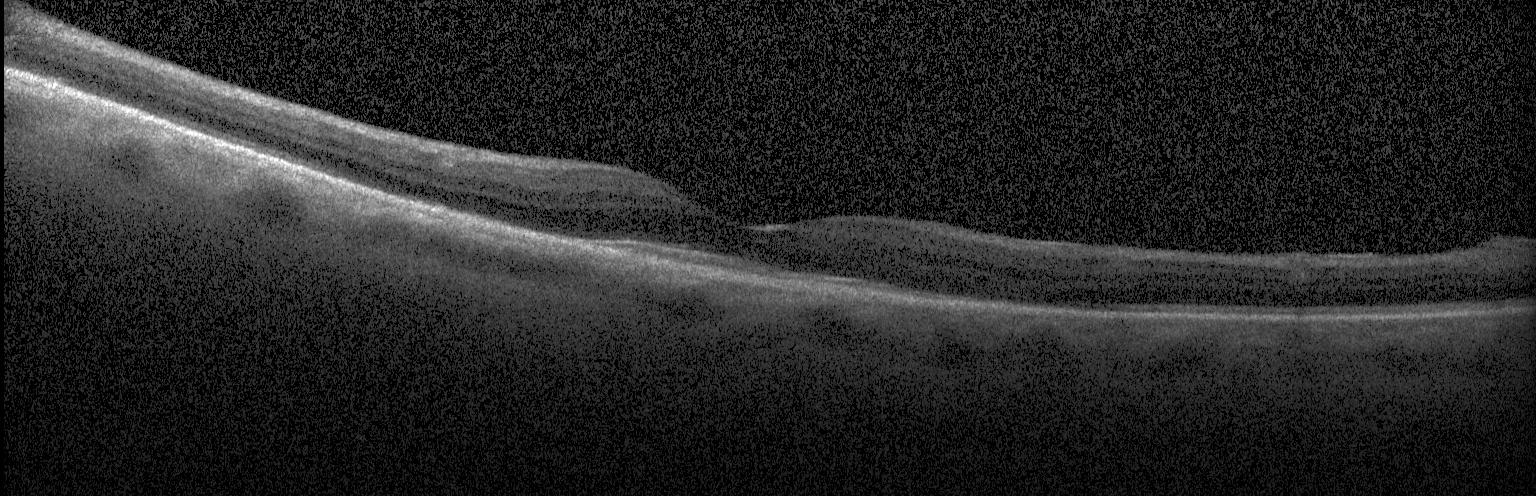
OCT B-scan — Impression: choroidal neovascularization.